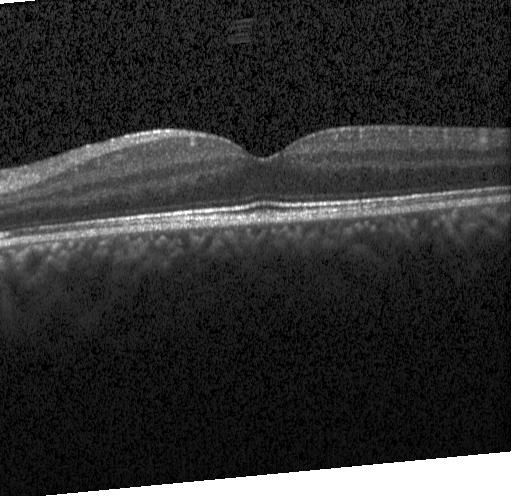
Assessment: no choroidal neovascularization, diabetic macular edema, or drusen.